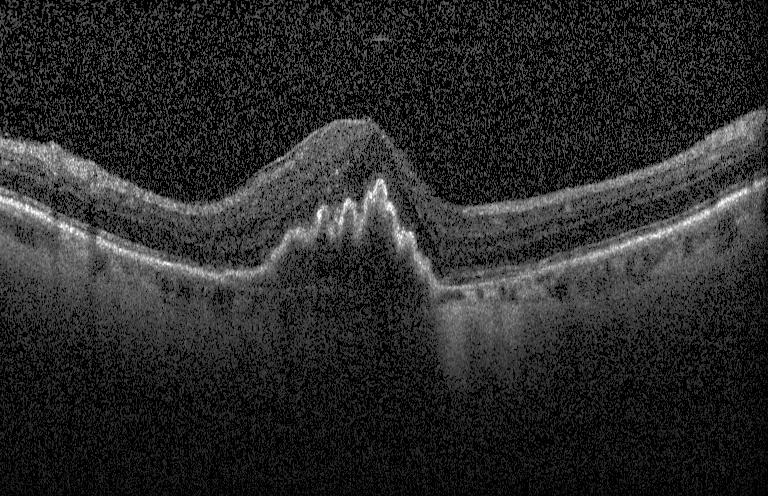

Acquired on a Heidelberg Spectralis · retinal OCT cross-section · macular scan · spectral-domain optical coherence tomography — OCT finding: choroidal neovascularization.